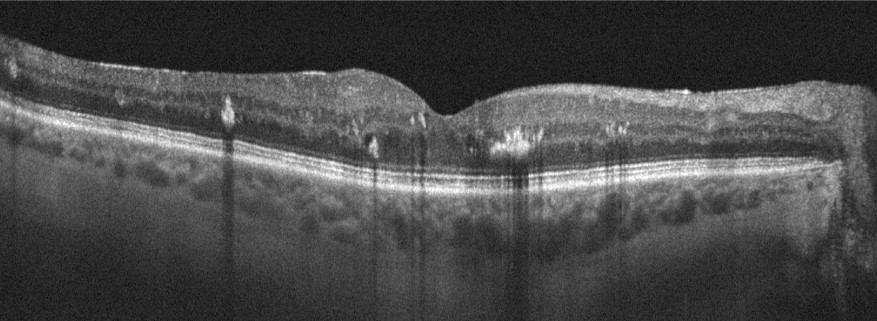 Finding: DME.